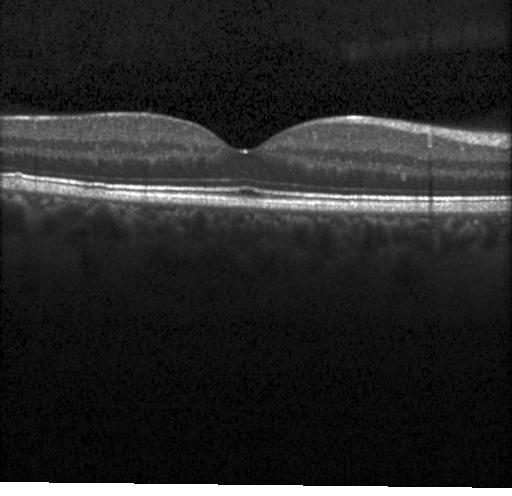 Spectral-domain OCT; OCT line scan
Macular OCT: no choroidal neovascularization, no diabetic macular edema, and no drusen.